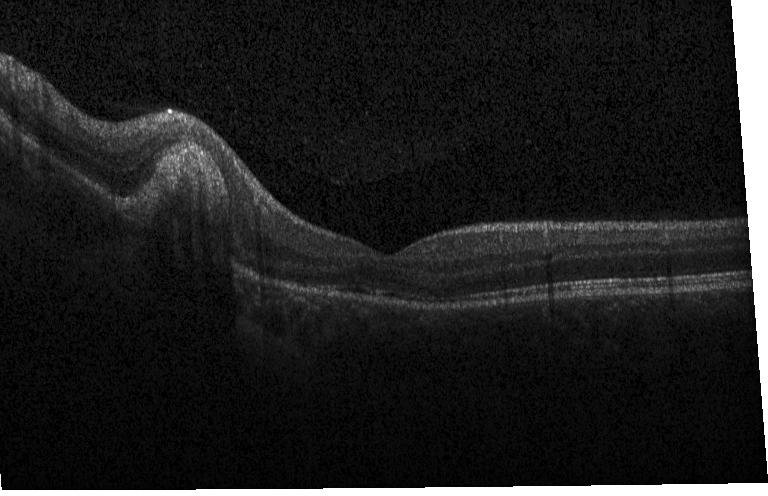
OCT line scan, SD-OCT.
Diagnosis: a choroidal neovascular membrane.